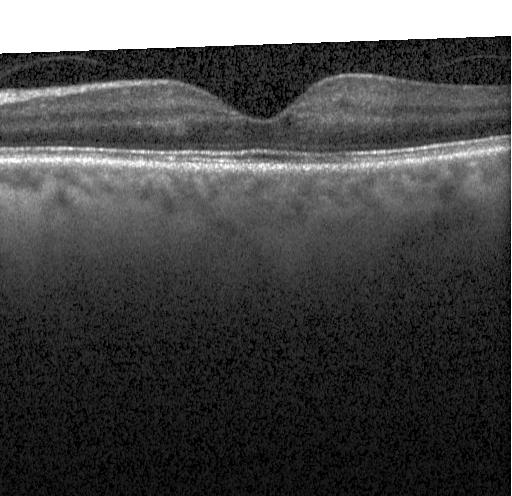

Dx: no choroidal neovascularization, no diabetic macular edema, and no drusen.